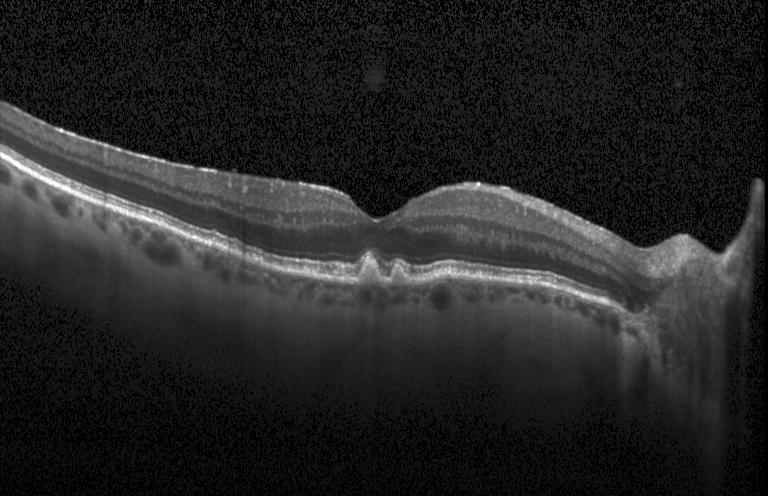 Optical coherence tomography B-scan — OCT finding: sub-RPE drusenoid deposits.